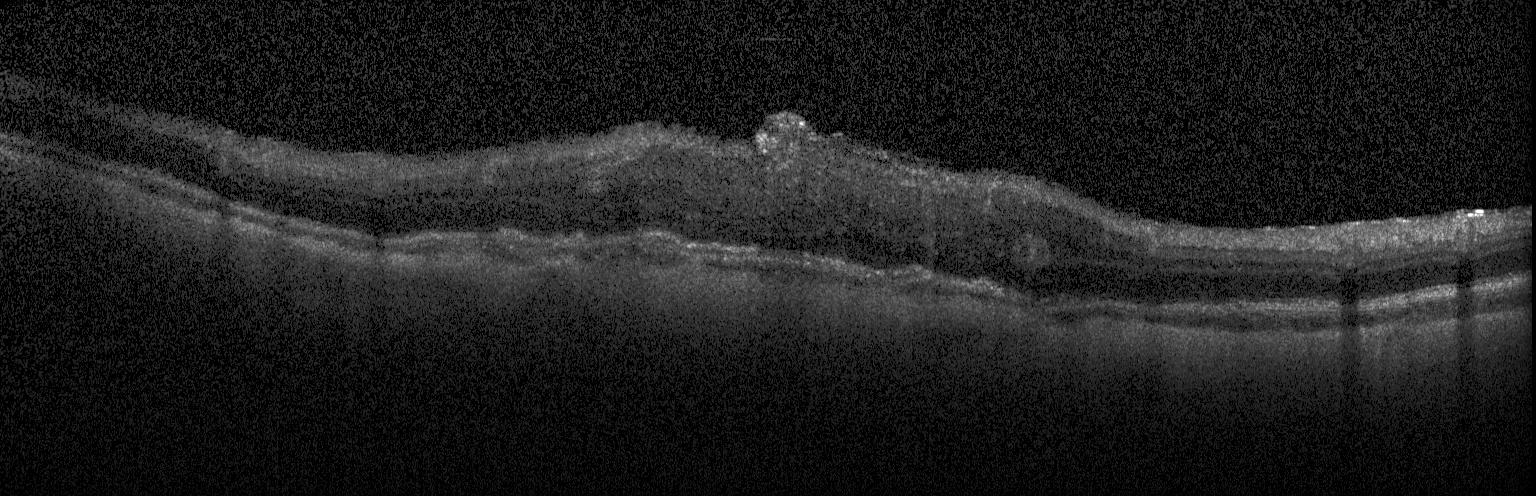
Retinal OCT cross-section; spectral-domain OCT; horizontal scan through the fovea
Diagnosis: diabetic macular edema.